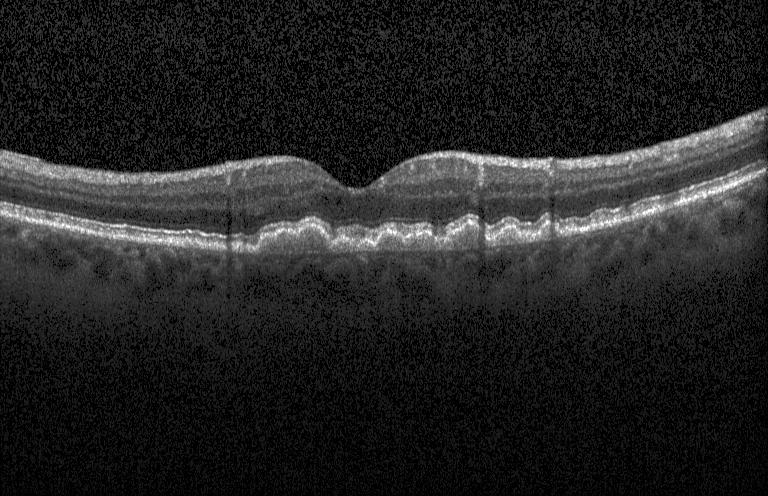
Retinal OCT B-scan · macular scan · acquired on a Heidelberg Spectralis — Finding: multiple drusen.